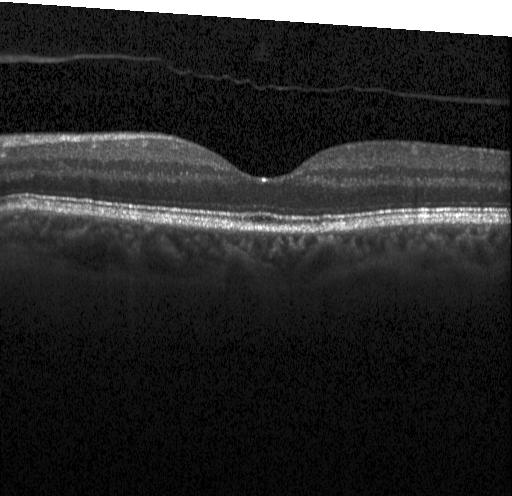

Diagnosis: no CNV, no DME, and no drusen.